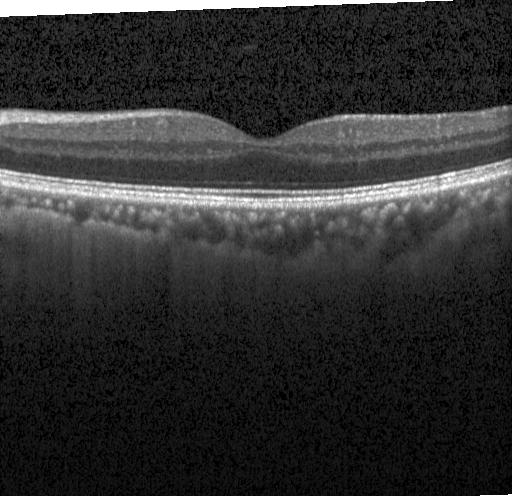 Retinal OCT cross-section showing no choroidal neovascularization, no diabetic macular edema, and no drusen.